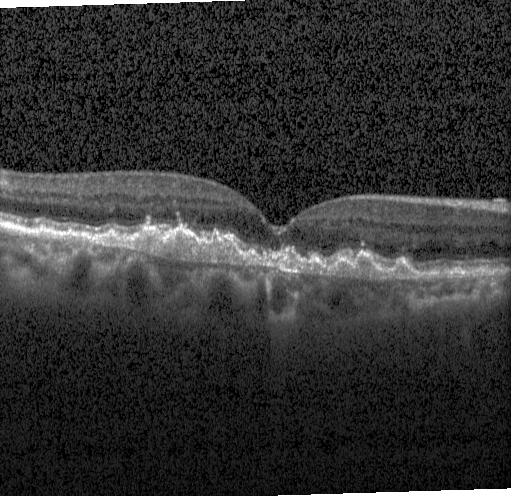 OCT B-scan. Assessment: a choroidal neovascular membrane.